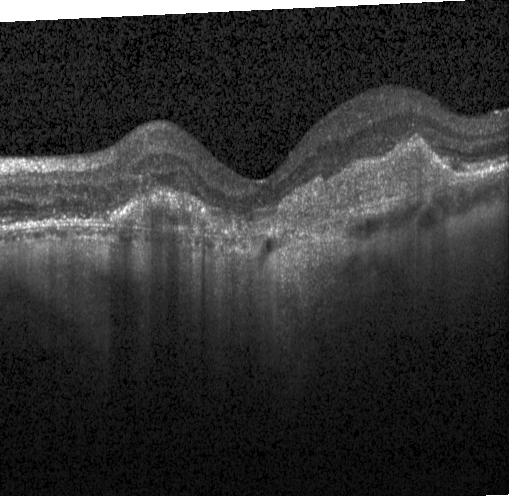

Spectral-domain OCT B-scan: a choroidal neovascular membrane.